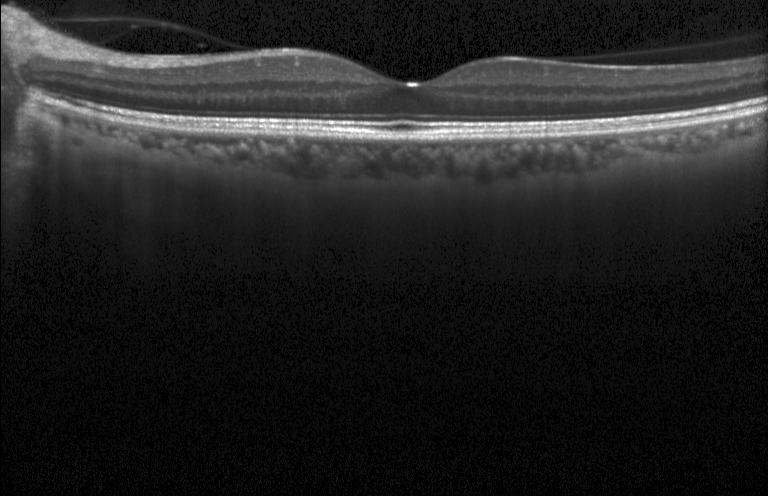

Centered on the fovea · acquired on a Heidelberg Spectralis · OCT B-scan
Diagnosis: no choroidal neovascularization, diabetic macular edema, or drusen.